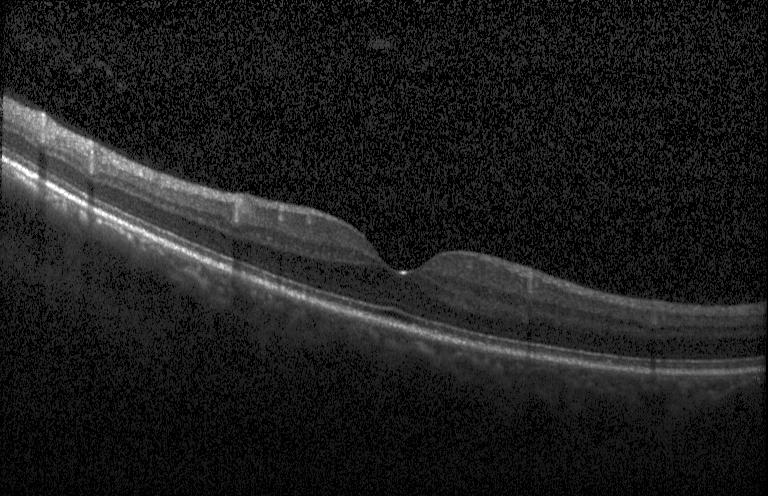 OCT finding: no evidence of choroidal neovascularization, diabetic macular edema, or drusen.